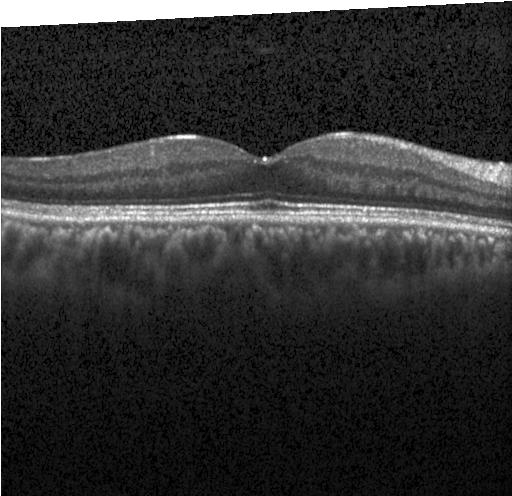 Retinal OCT B-scan, instrument: Heidelberg Spectralis, spectral-domain optical coherence tomography
Dx: no evidence of choroidal neovascularization, diabetic macular edema, or drusen.